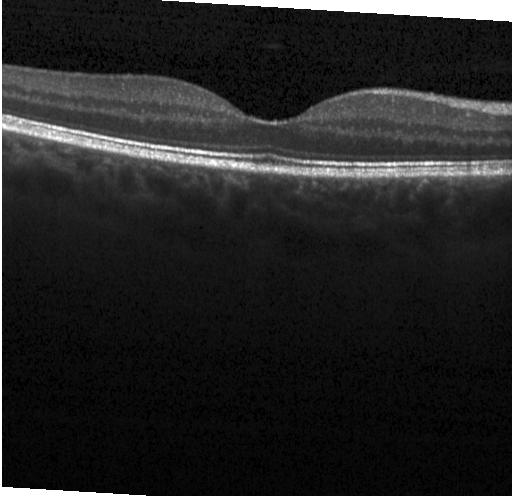

Diagnosis: neither choroidal neovascularization, diabetic macular edema, nor drusen.